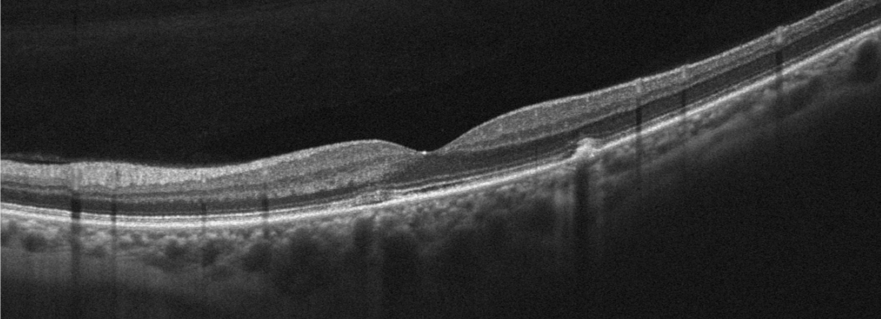

Macular scan · OCT line scan. Assessment: age-related macular degeneration (AMD).